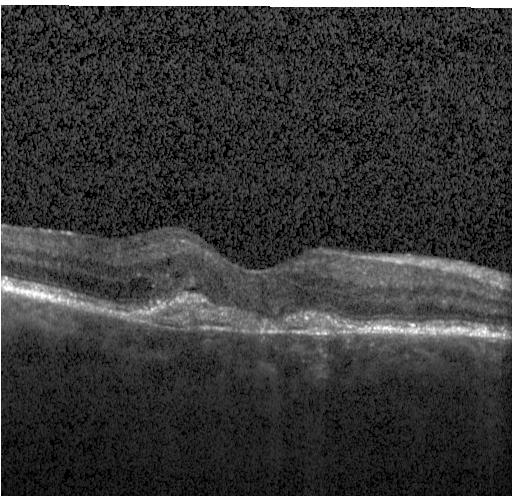 OCT B-scan — This B-scan demonstrates CNV.